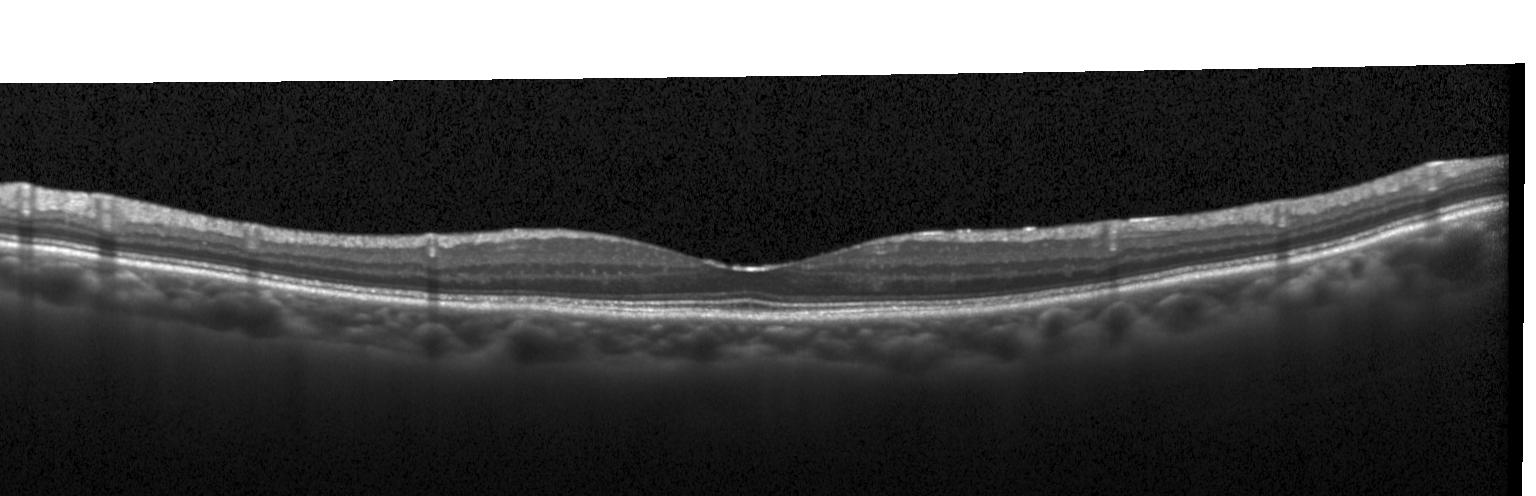
OCT line scan
OCT finding: neither CNV, DME, nor drusen.